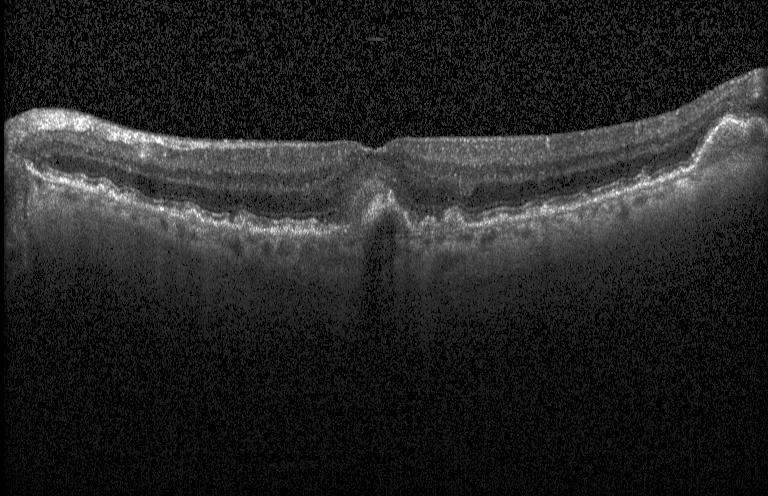

Impression: choroidal neovascularization.